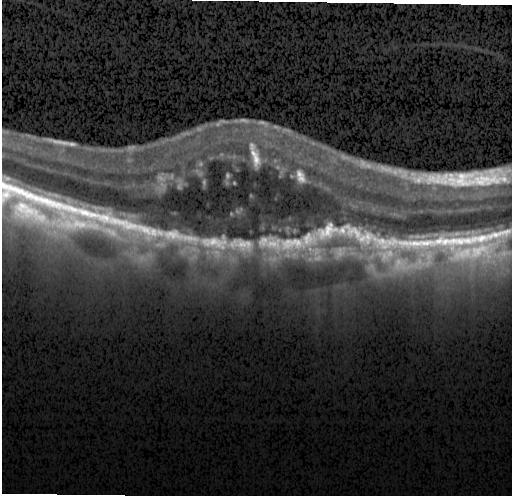

Optical coherence tomography scan, acquired on a Heidelberg Spectralis.
Assessment: choroidal neovascularization.